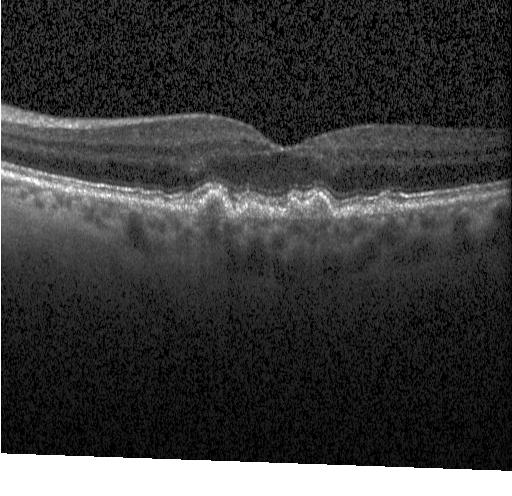

Instrument: Heidelberg Spectralis. SD-OCT. Optical coherence tomography B-scan. Horizontal scan through the fovea. The scan shows drusen.